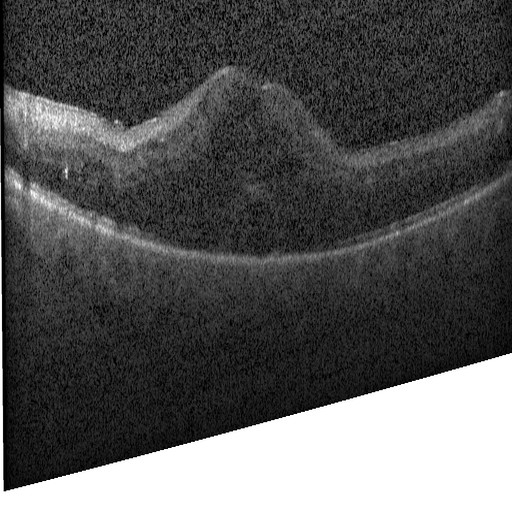
Optical coherence tomography scan, centered on the fovea, spectral-domain optical coherence tomography
Impression: diabetic macular edema.